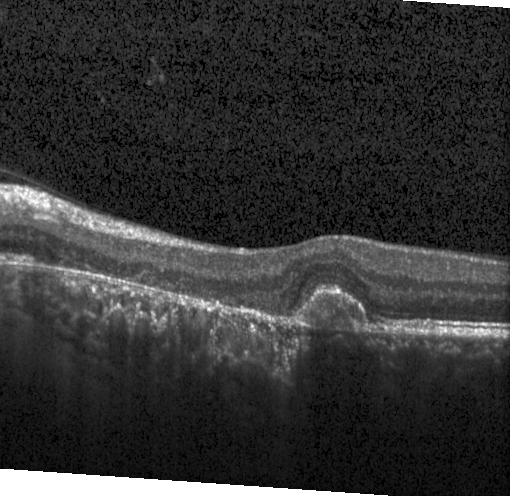 Finding: a choroidal neovascular membrane.